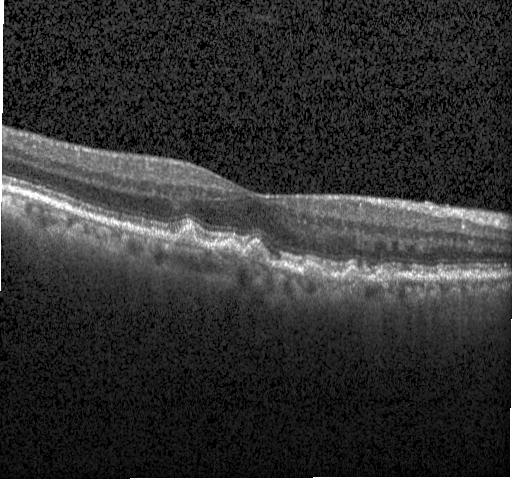 Through the macula, acquired on a Heidelberg Spectralis, SD-OCT, retinal OCT B-scan — Finding: multiple drusen.